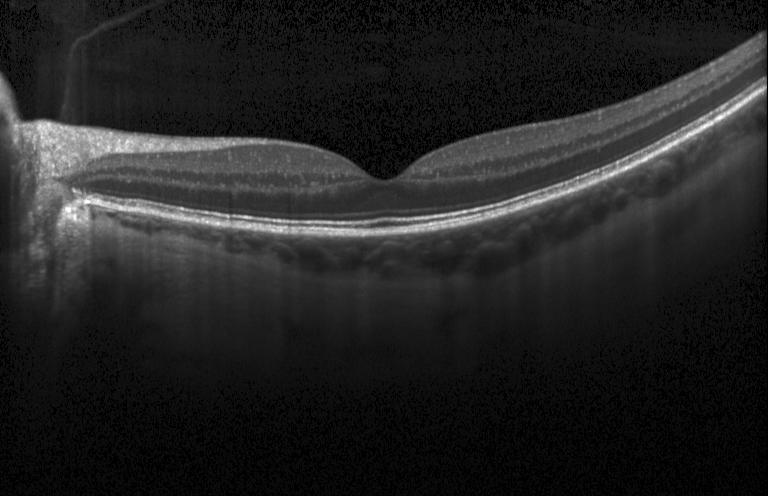

Retinal OCT B-scan. Horizontal scan through the fovea
OCT finding: neither CNV, DME, nor drusen.